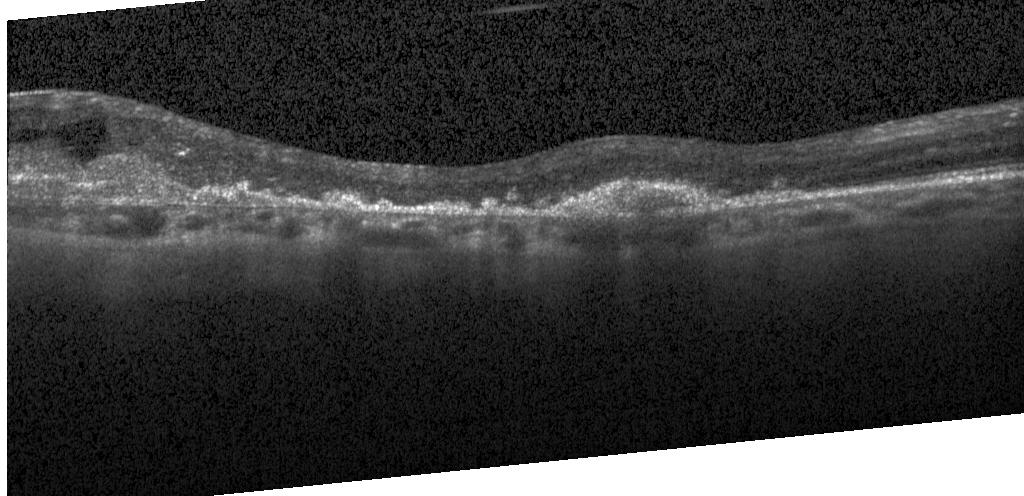
Macular OCT demonstrating CNV.